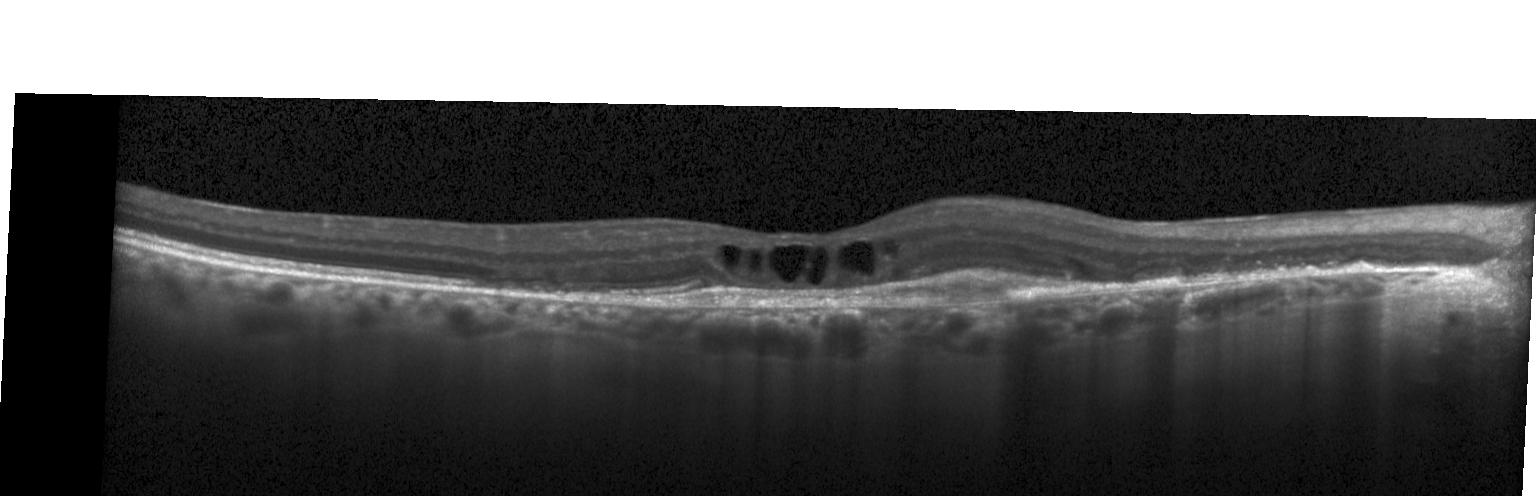
Horizontal scan through the fovea, optical coherence tomography B-scan.
Assessment: a choroidal neovascular membrane.